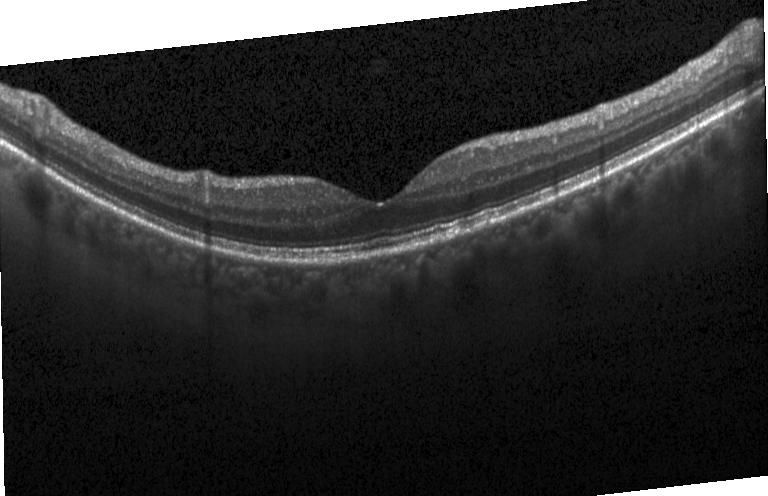 OCT B-scan. Spectral-domain optical coherence tomography. Horizontal scan through the fovea. Heidelberg Spectralis OCT system.
Diagnosis: no choroidal neovascularization, diabetic macular edema, or drusen.